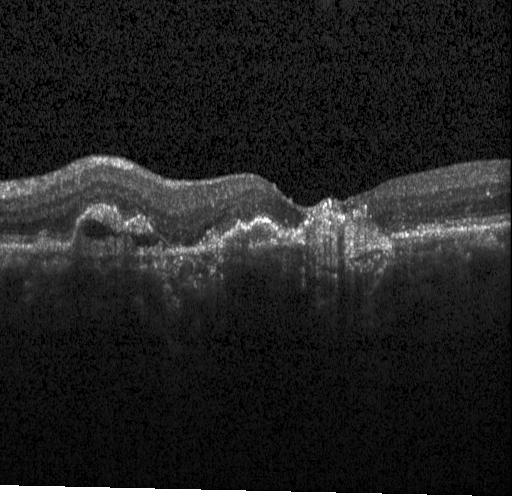
Spectral-domain optical coherence tomography · retinal OCT B-scan · horizontal scan through the fovea. Finding: a choroidal neovascular membrane.